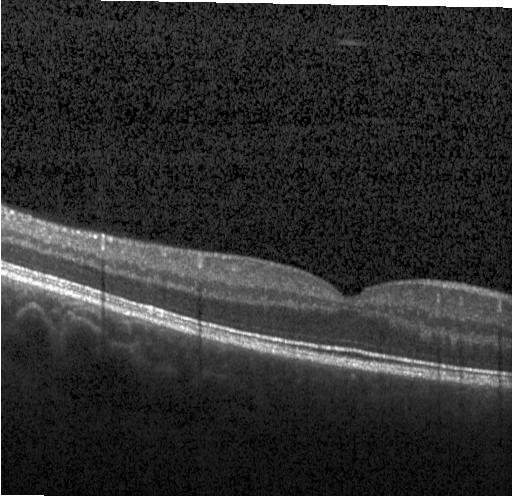

No evidence of choroidal neovascularization, diabetic macular edema, or drusen.